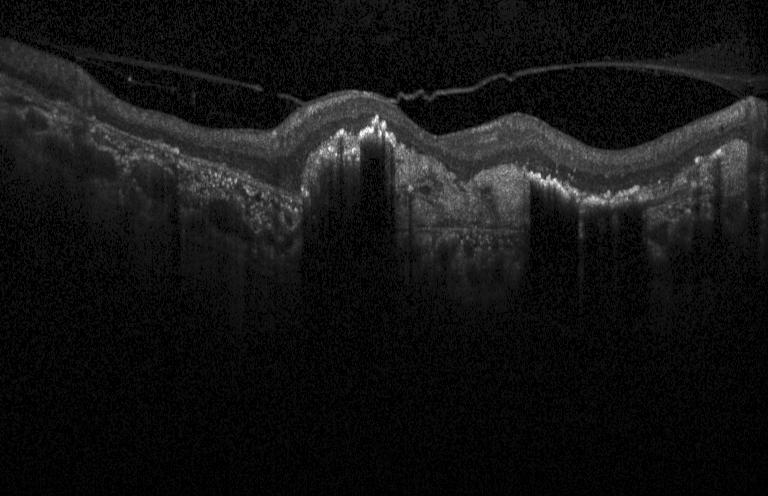
Spectral-domain optical coherence tomography · fovea-centered · optical coherence tomography B-scan · acquired on a Heidelberg Spectralis.
Diagnosis: a choroidal neovascular membrane.